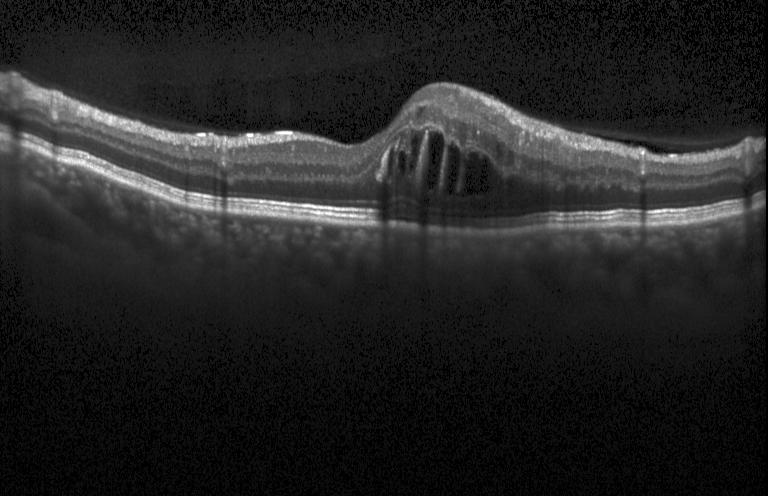
OCT B-scan showing DME.